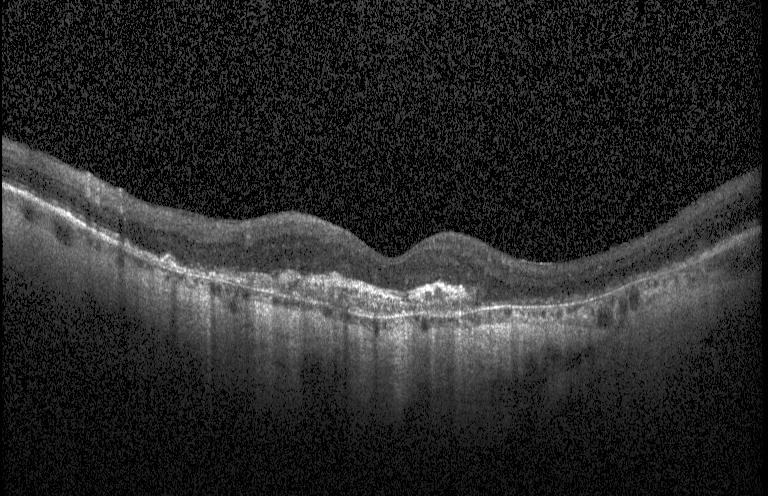
OCT finding: a choroidal neovascular membrane.